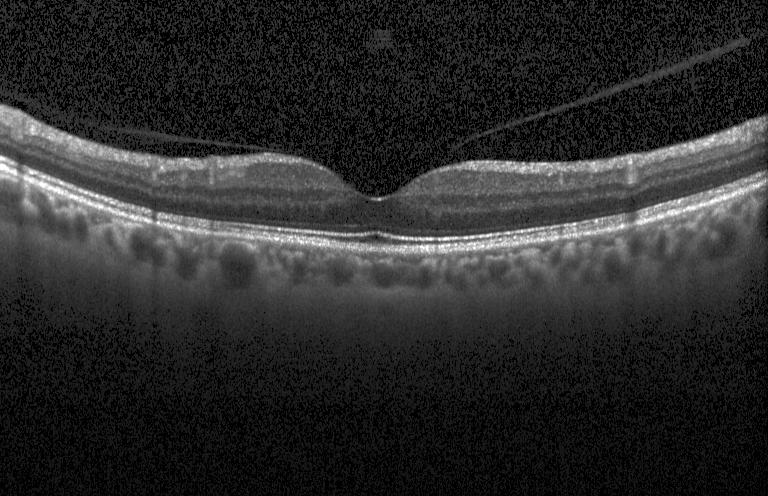

Horizontal scan through the fovea, Heidelberg Spectralis OCT system, retinal OCT B-scan, SD-OCT.
Macular OCT: neither choroidal neovascularization, diabetic macular edema, nor drusen.